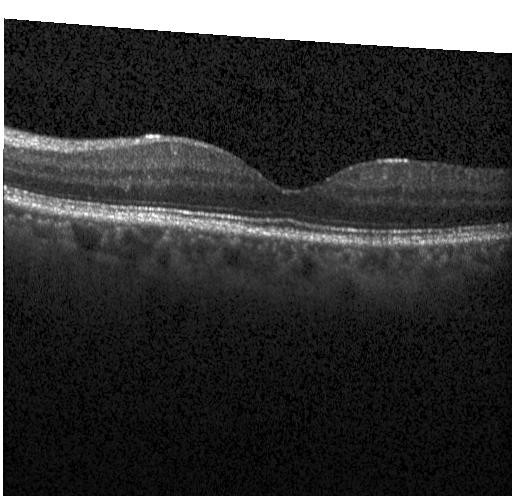 Spectral-domain optical coherence tomography. Optical coherence tomography B-scan. The scan shows no choroidal neovascularization, no diabetic macular edema, and no drusen.